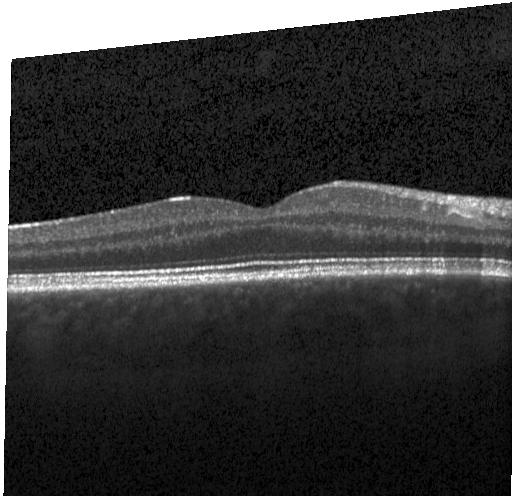
OCT line scan — Assessment: no choroidal neovascularization, diabetic macular edema, or drusen.